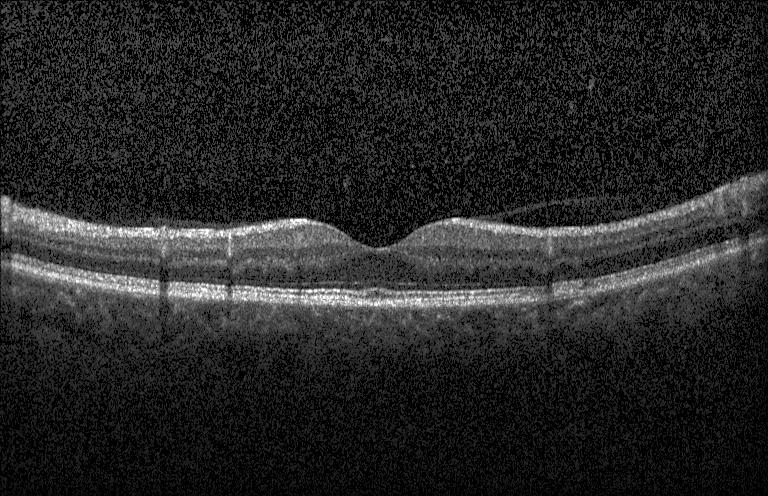
Fovea-centered, retinal OCT cross-section, spectral-domain optical coherence tomography. Impression: neither choroidal neovascularization, diabetic macular edema, nor drusen.